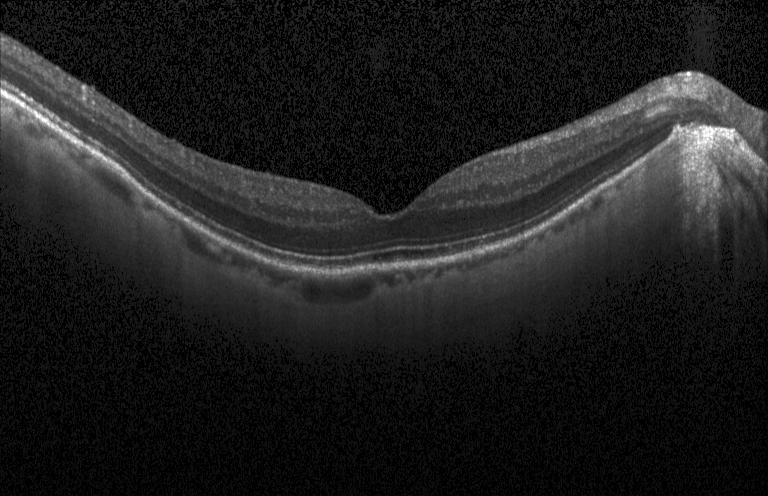 OCT B-scan showing no CNV, no DME, and no drusen.